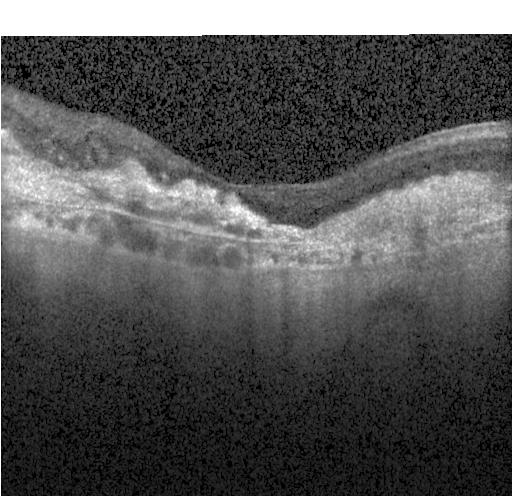

Heidelberg Spectralis OCT system. Spectral-domain OCT. Fovea-centered. Optical coherence tomography B-scan.
Assessment: a choroidal neovascular membrane.